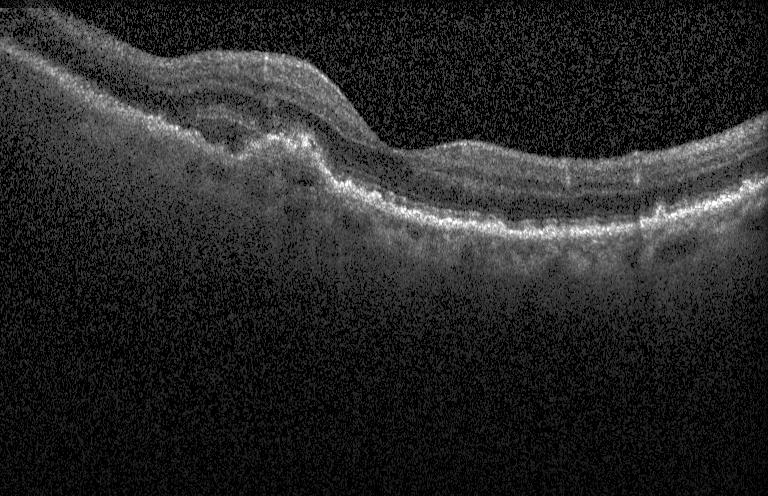 Finding: a choroidal neovascular membrane.